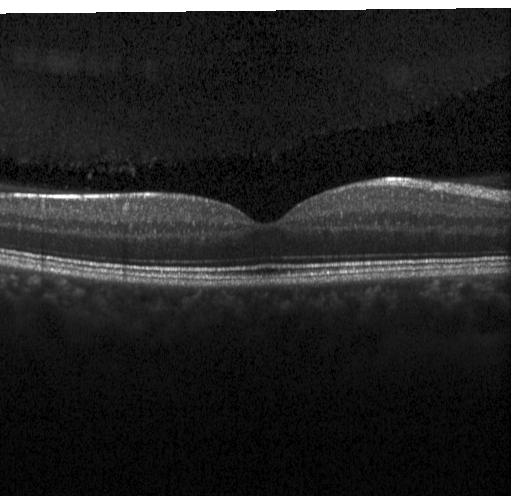 Impression: no choroidal neovascularization, no diabetic macular edema, and no drusen.